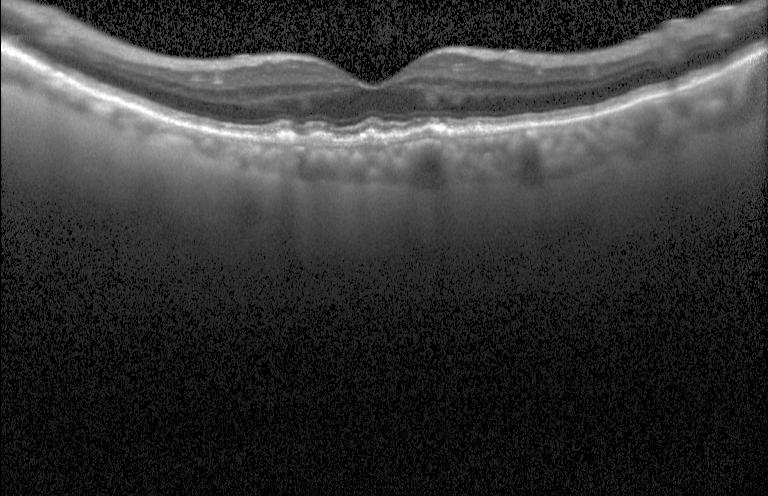
OCT B-scan.
Impression: drusen.